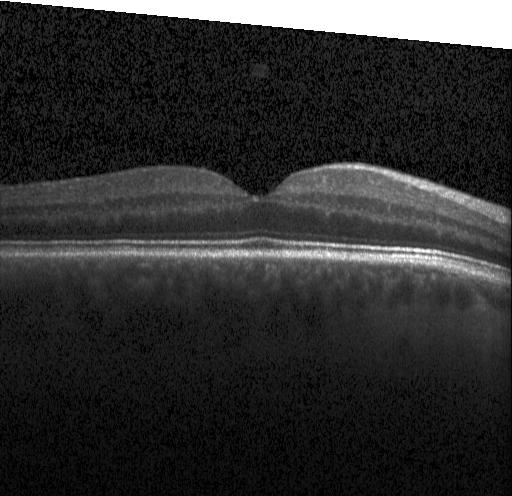

Retinal OCT cross-section. Heidelberg Spectralis OCT system. OCT finding: no choroidal neovascularization, no diabetic macular edema, and no drusen.